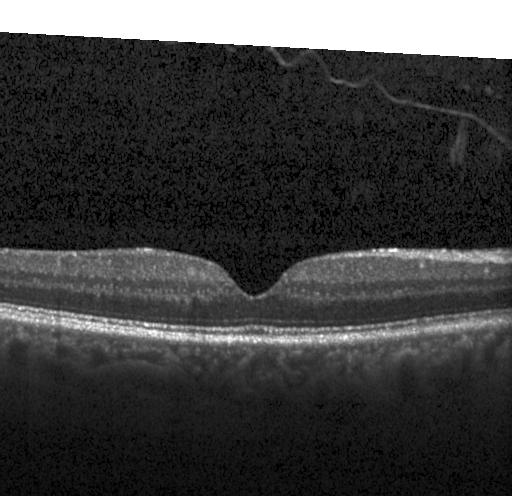 Horizontal scan through the fovea, OCT B-scan, SD-OCT
The scan shows neither choroidal neovascularization, diabetic macular edema, nor drusen.